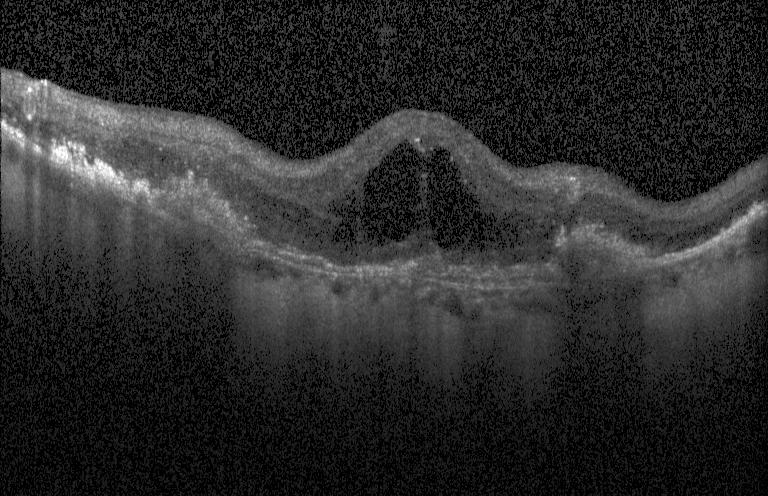 Retinal OCT cross-section
Choroidal neovascularization.